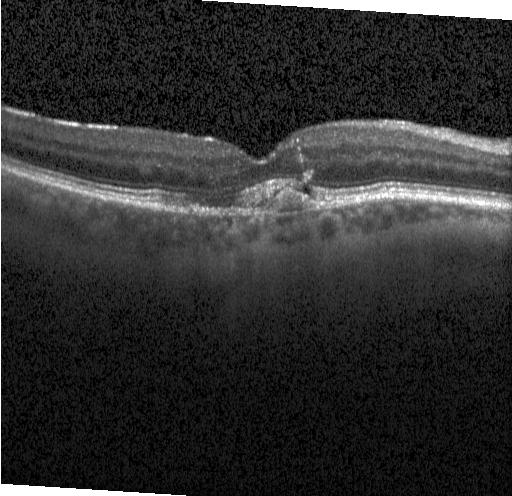

OCT B-scan · spectral-domain OCT · acquired on a Heidelberg Spectralis · macular scan
Choroidal neovascularization (CNV).